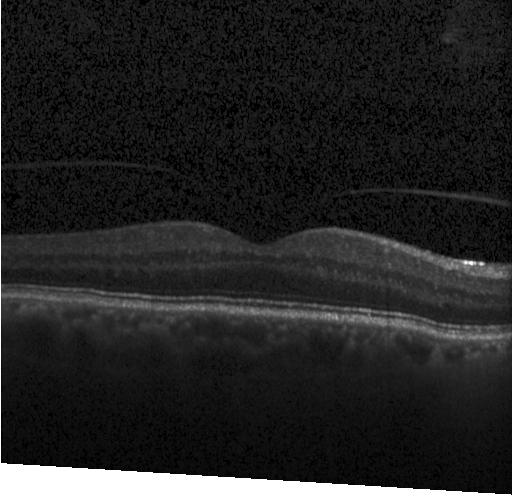
OCT line scan
Diagnosis: no CNV, DME, or drusen.